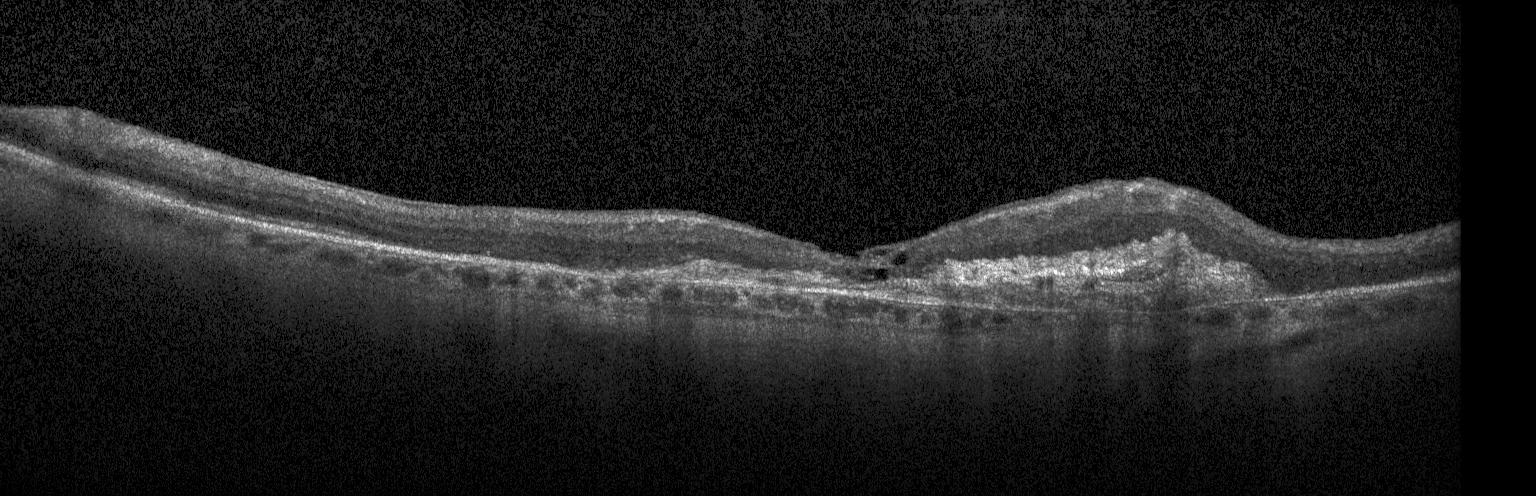

Spectral-domain OCT; through the macula; optical coherence tomography B-scan
This B-scan demonstrates choroidal neovascularization (CNV).